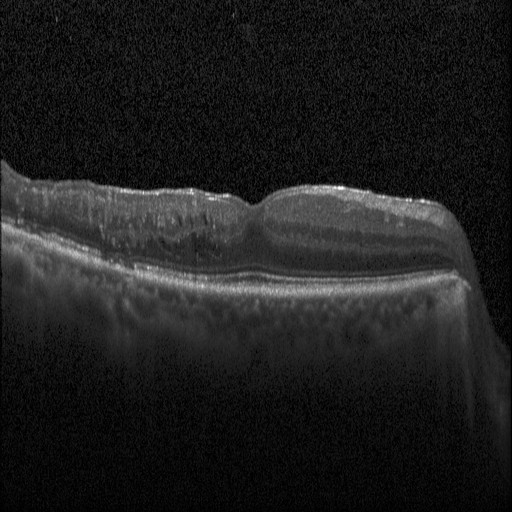

OCT B-scan · centered on the fovea
Impression: diabetic macular edema.